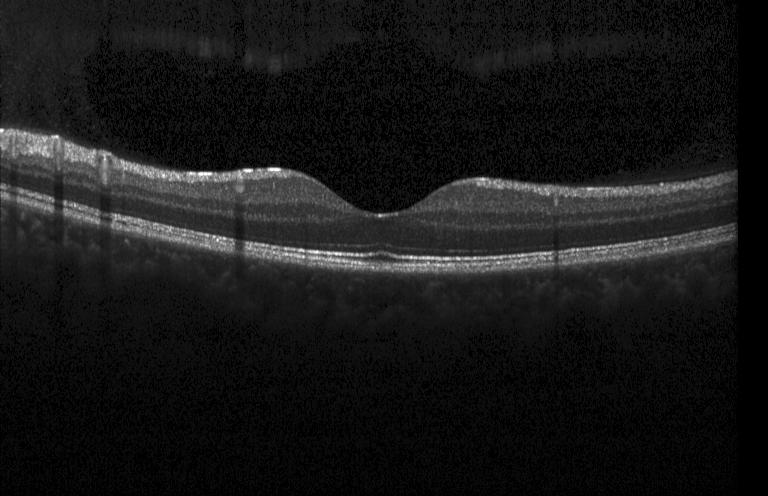

Spectral-domain OCT B-scan: no CNV, no DME, and no drusen.